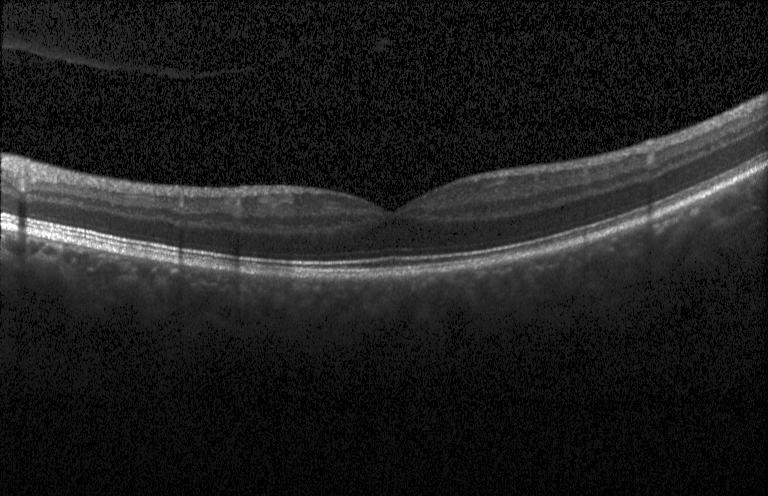

Optical coherence tomography B-scan · spectral-domain OCT — Finding: no CNV, no DME, and no drusen.